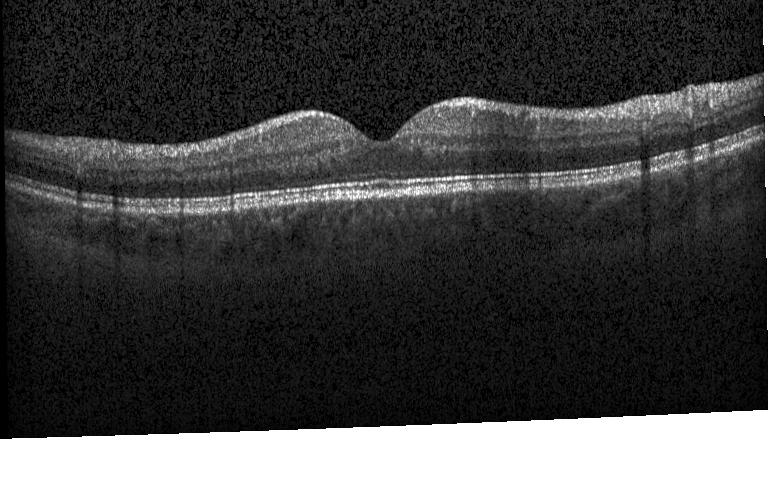 Acquired on a Heidelberg Spectralis, fovea-centered, spectral-domain OCT, optical coherence tomography B-scan
Impression: no CNV, DME, or drusen.